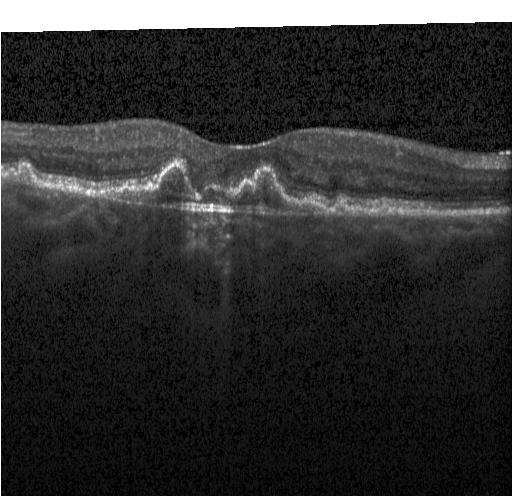

Heidelberg Spectralis · OCT line scan · spectral-domain OCT · macular scan. A choroidal neovascular membrane.